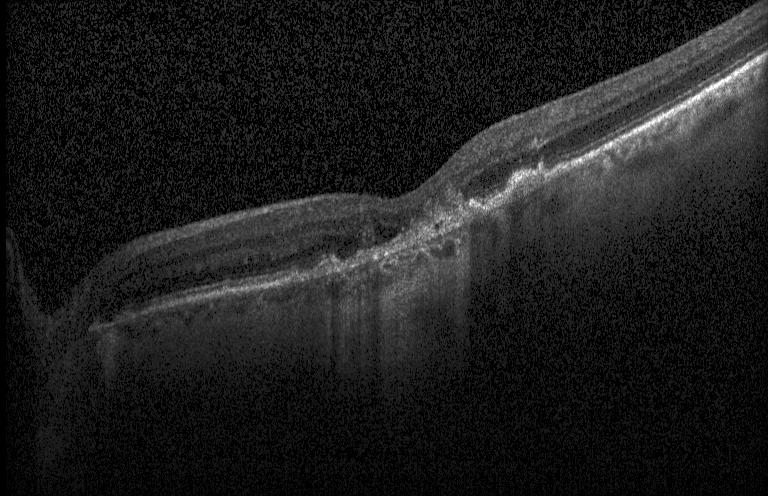

Macular OCT: choroidal neovascularization (CNV).